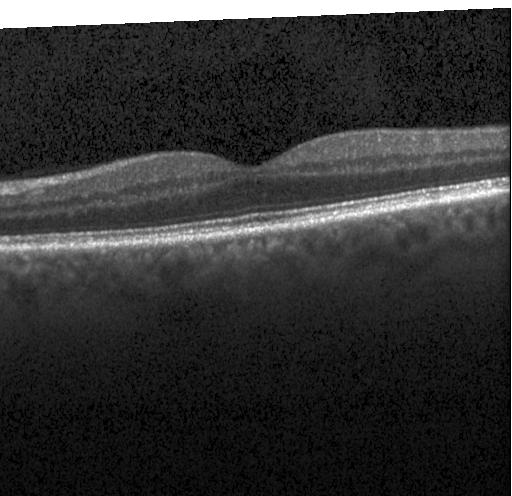 Impression: no choroidal neovascularization, diabetic macular edema, or drusen.